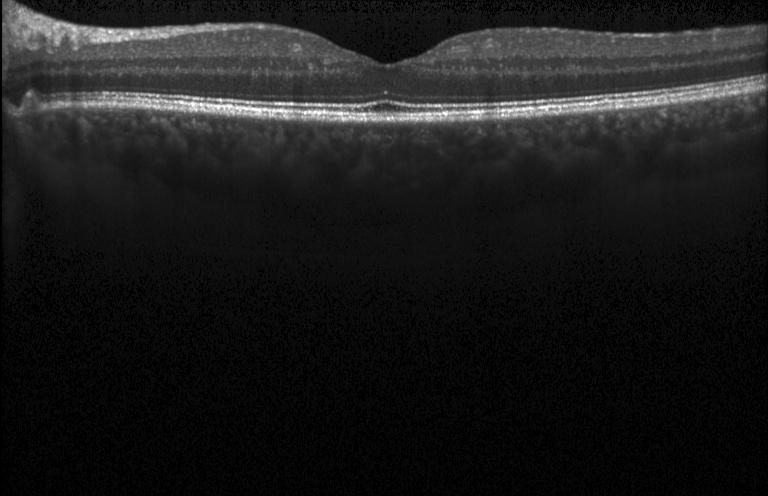

Spectral-domain OCT B-scan: no choroidal neovascularization, no diabetic macular edema, and no drusen.